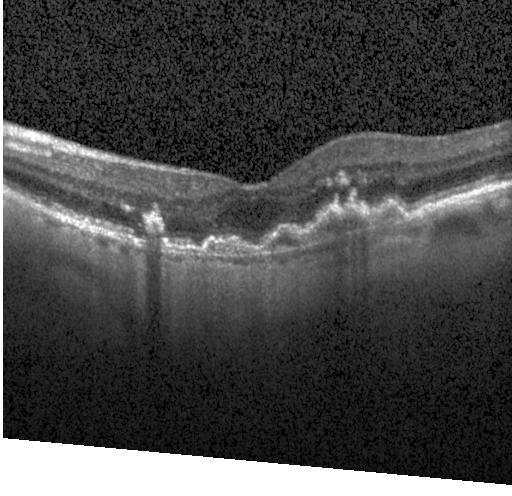

Finding: CNV.